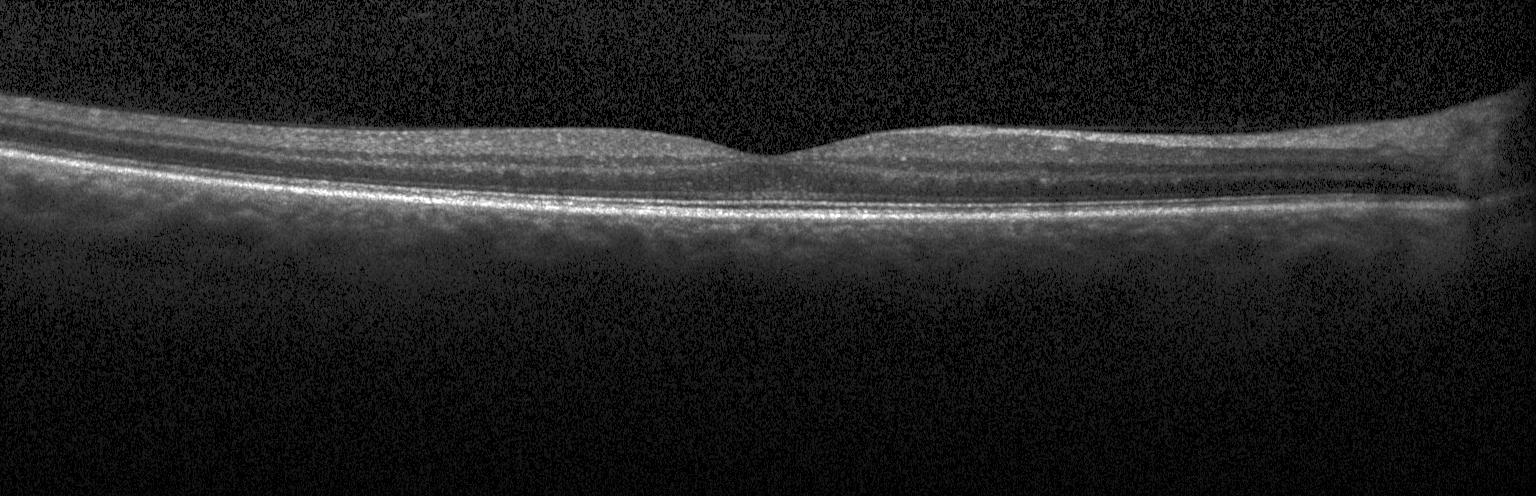 No CNV, DME, or drusen.